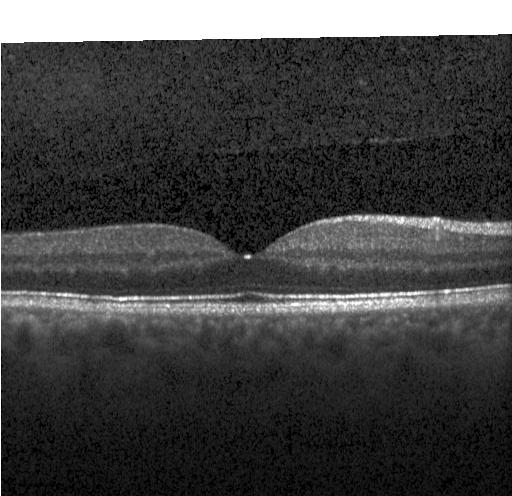

Optical coherence tomography B-scan
Dx: no choroidal neovascularization, no diabetic macular edema, and no drusen.